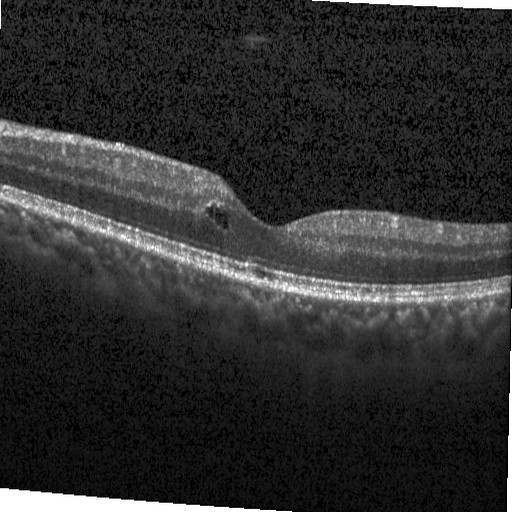
Spectral-domain OCT; OCT B-scan.
Finding: diabetic macular edema (DME).